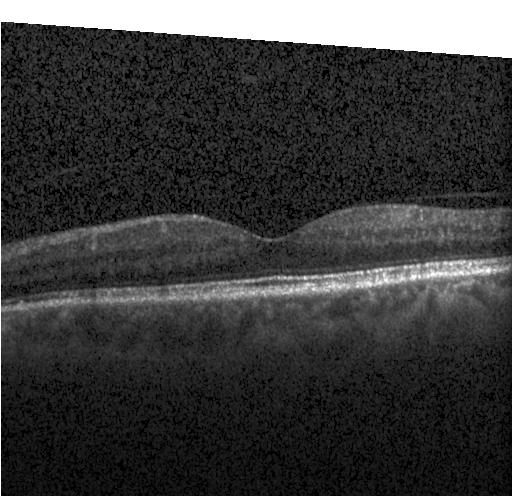 Horizontal scan through the fovea. Spectral-domain OCT. OCT line scan. Heidelberg Spectralis OCT system
This B-scan demonstrates no evidence of CNV, DME, or drusen.